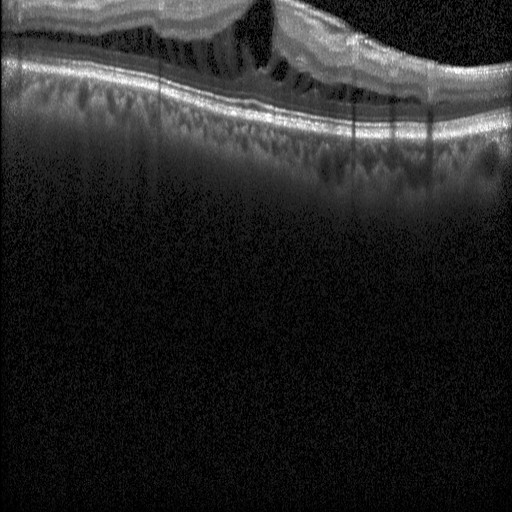

DME.